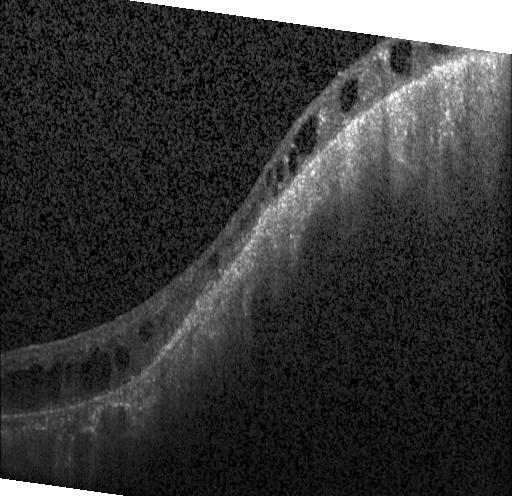 Dx: DME.